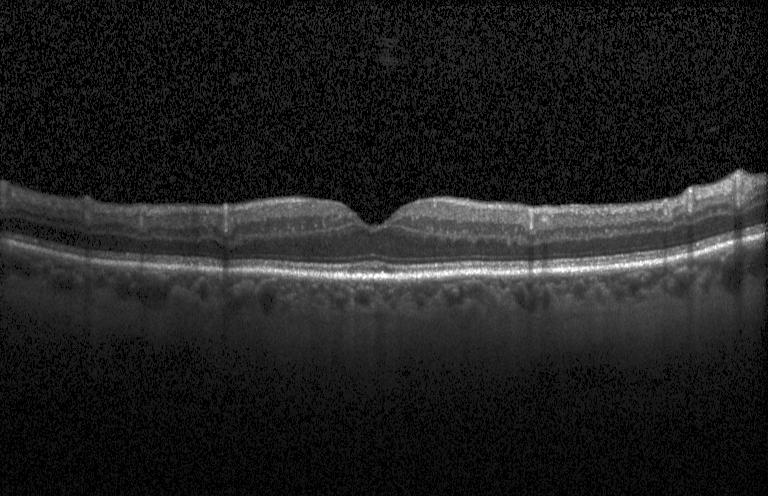

Spectral-domain optical coherence tomography · OCT line scan. Finding: no CNV, DME, or drusen.